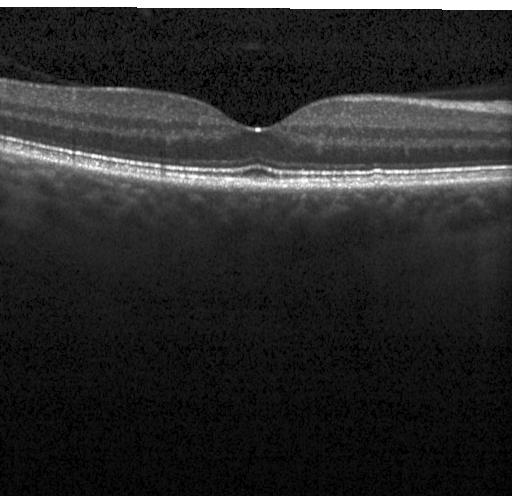 Impression: no evidence of choroidal neovascularization, diabetic macular edema, or drusen.